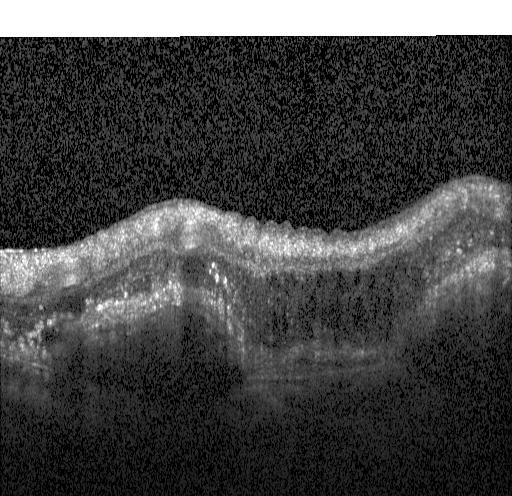 Macular OCT demonstrating CNV.